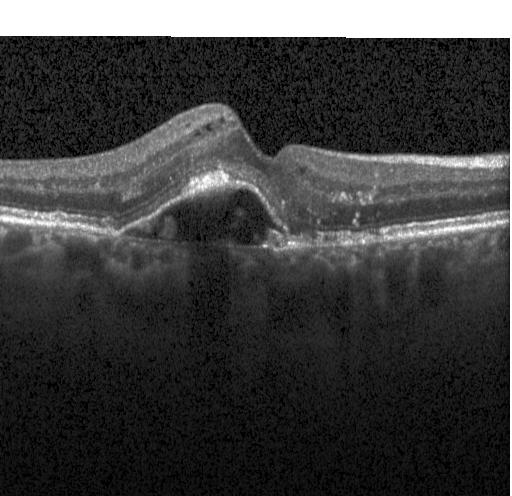
Spectral-domain OCT; optical coherence tomography scan; fovea-centered; instrument: Heidelberg Spectralis — This B-scan demonstrates choroidal neovascularization.